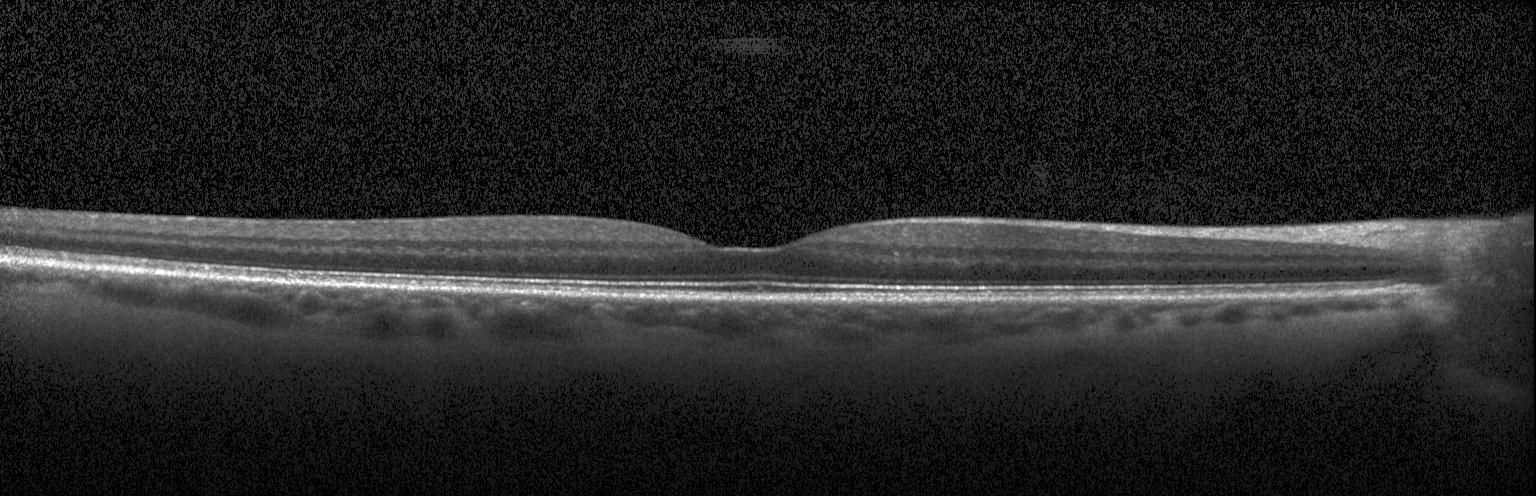
Horizontal scan through the fovea · OCT line scan
Diagnosis: no CNV, DME, or drusen.